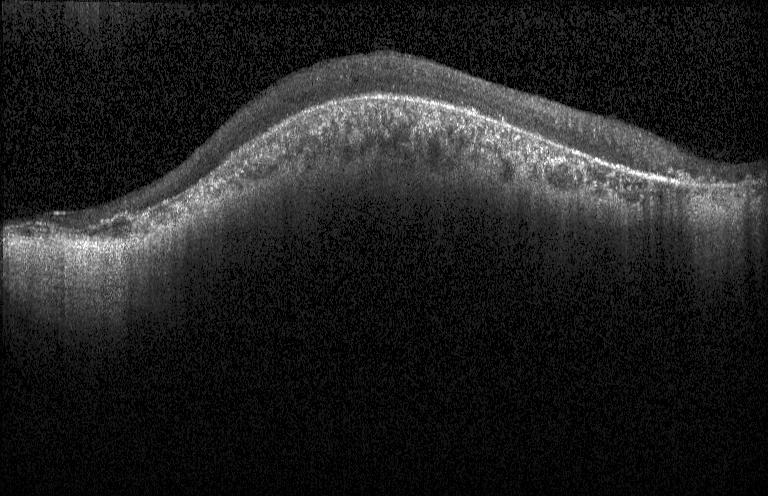

Impression: no choroidal neovascularization, no diabetic macular edema, and no drusen.